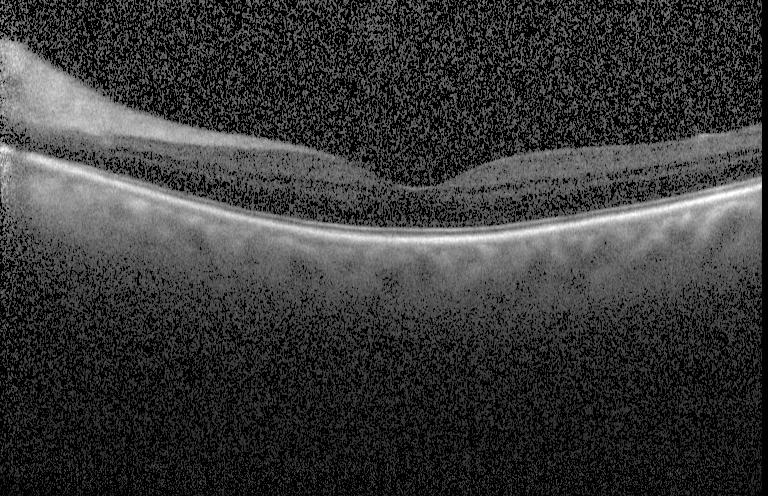 Spectral-domain optical coherence tomography. OCT B-scan. Instrument: Heidelberg Spectralis. Horizontal scan through the fovea.
Neither choroidal neovascularization, diabetic macular edema, nor drusen.